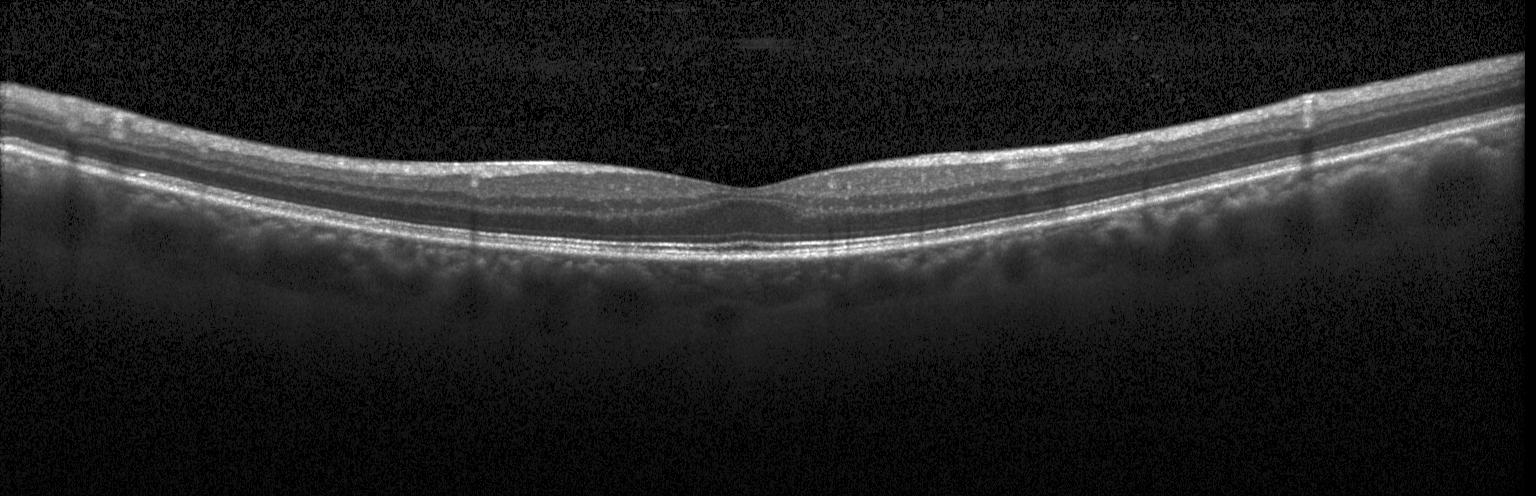 SD-OCT. Optical coherence tomography scan. Horizontal scan through the fovea. Instrument: Heidelberg Spectralis. Assessment: neither choroidal neovascularization, diabetic macular edema, nor drusen.